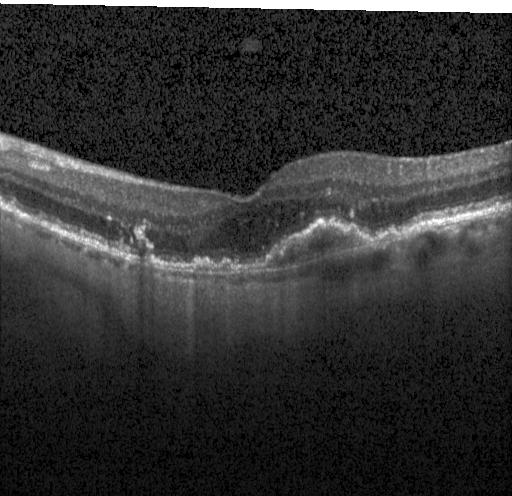 Optical coherence tomography scan; spectral-domain OCT — Diagnosis: a choroidal neovascular membrane.